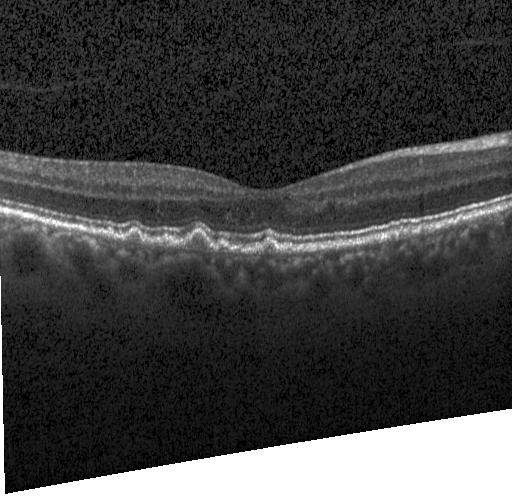

Spectral-domain optical coherence tomography · Heidelberg Spectralis OCT system · retinal OCT cross-section. Dx: multiple drusen.